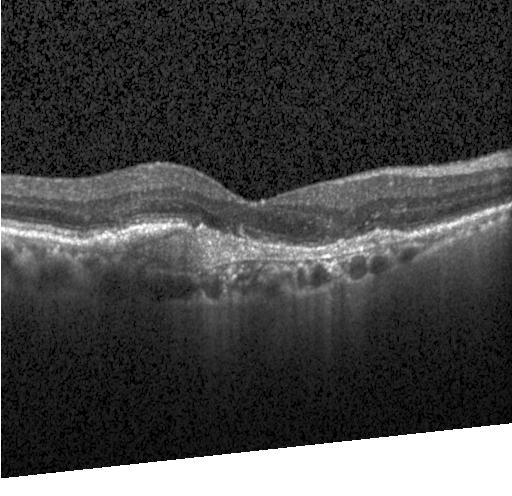 Diagnosis: a choroidal neovascular membrane.